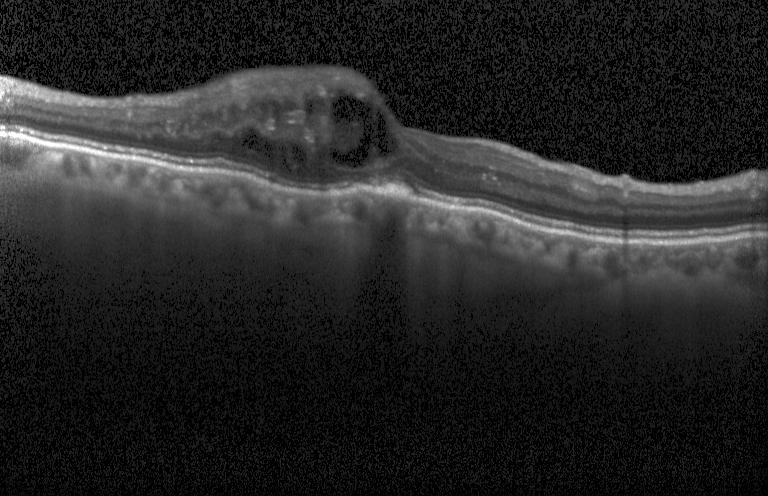
Optical coherence tomography scan. Spectral-domain optical coherence tomography. Horizontal scan through the fovea
Assessment: diabetic macular edema.